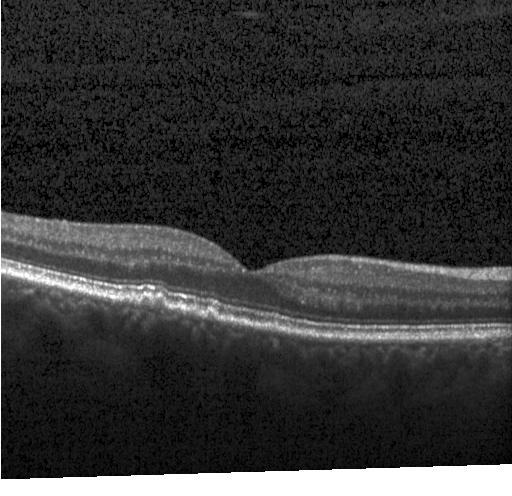

Fovea-centered. Optical coherence tomography scan. Finding: drusen.